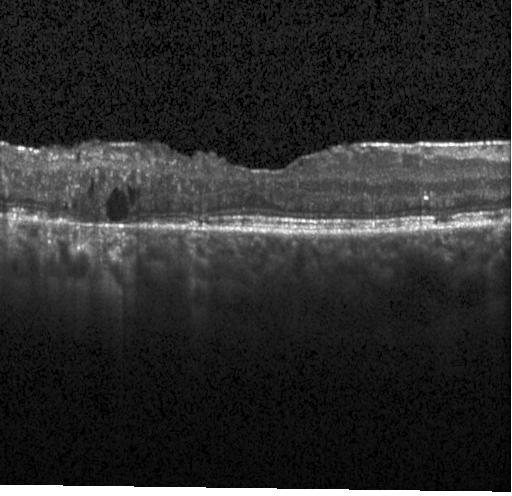 Optical coherence tomography B-scan. Acquired on a Heidelberg Spectralis. Through the macula — The scan shows diabetic macular edema (DME).